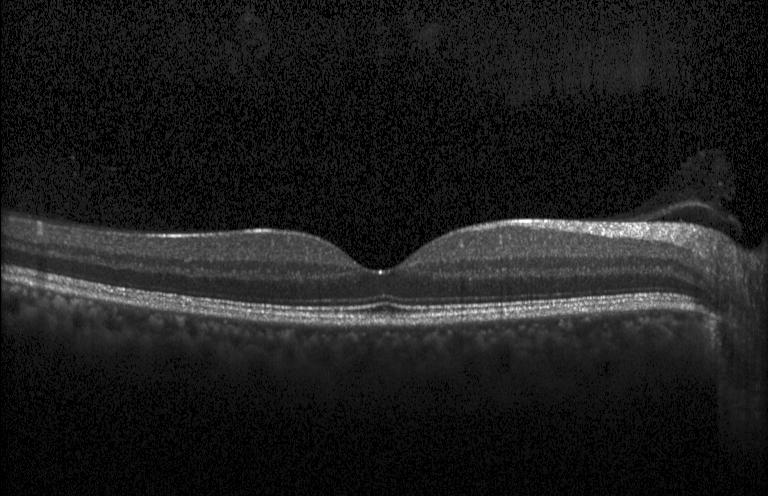 Finding: no evidence of choroidal neovascularization, diabetic macular edema, or drusen.